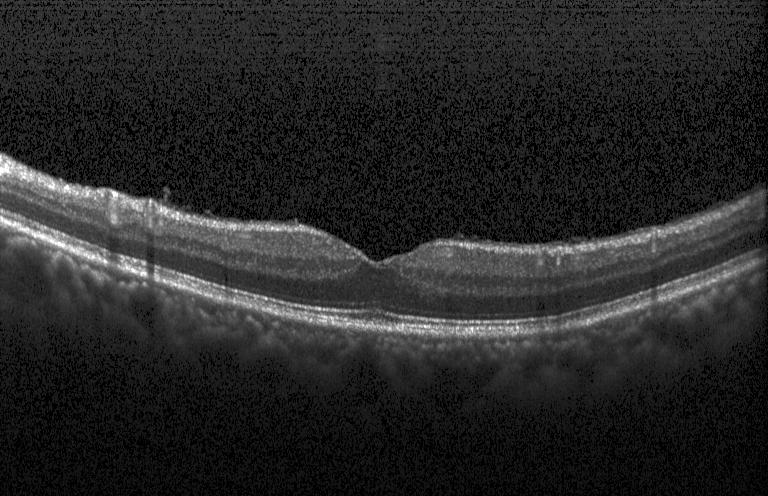

OCT scan showing no evidence of choroidal neovascularization, diabetic macular edema, or drusen.